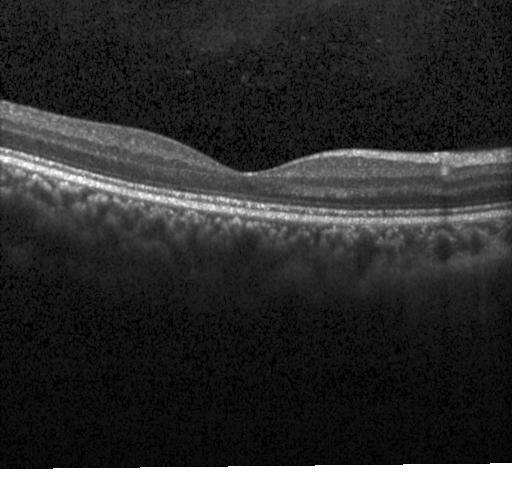

Retinal OCT B-scan — Macular OCT: no CNV, DME, or drusen.